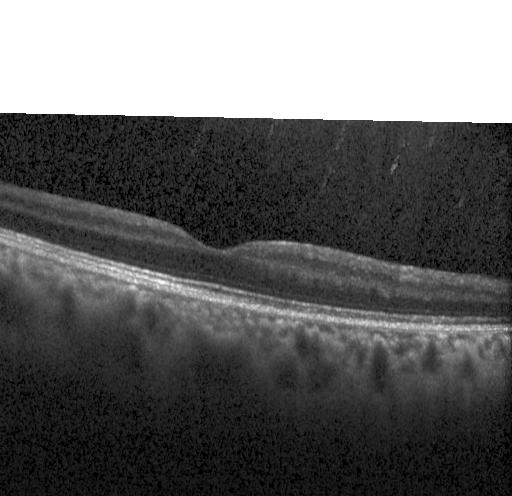

Fovea-centered · optical coherence tomography scan.
Impression: no evidence of CNV, DME, or drusen.